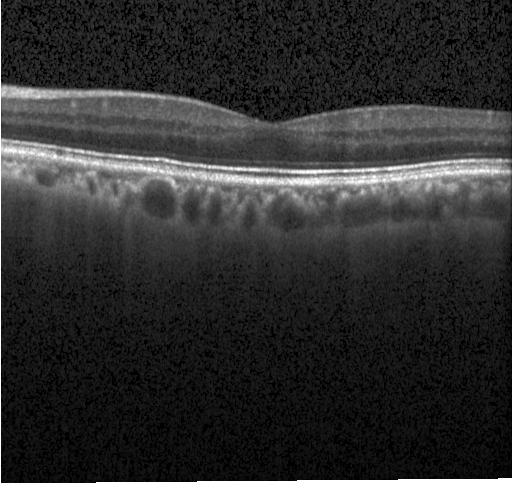

OCT B-scan
The scan shows no choroidal neovascularization, no diabetic macular edema, and no drusen.